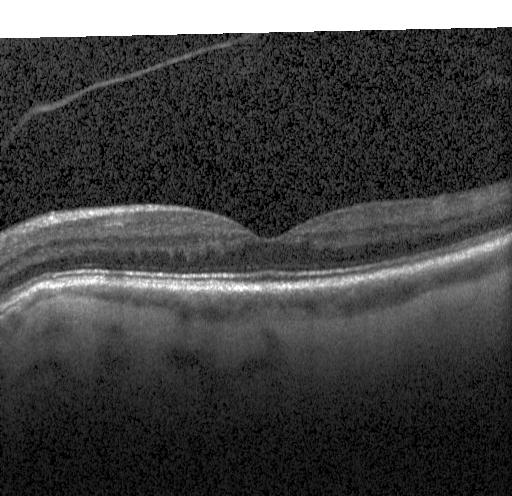

Retinal OCT B-scan. Through the macula — Assessment: no evidence of CNV, DME, or drusen.